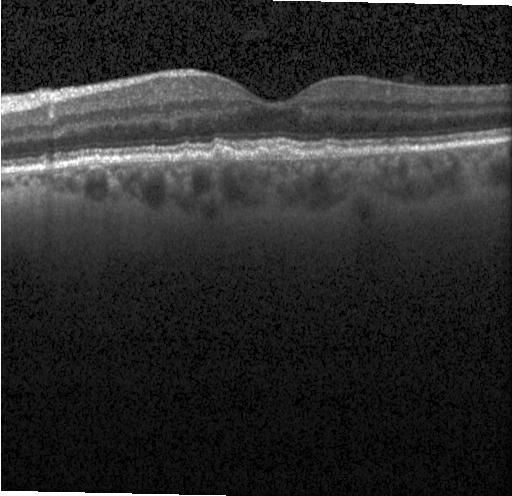
OCT scan showing multiple drusen.